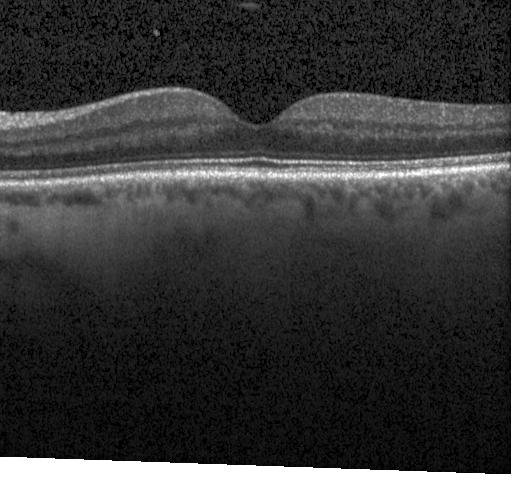
Diagnosis: no choroidal neovascularization, no diabetic macular edema, and no drusen.